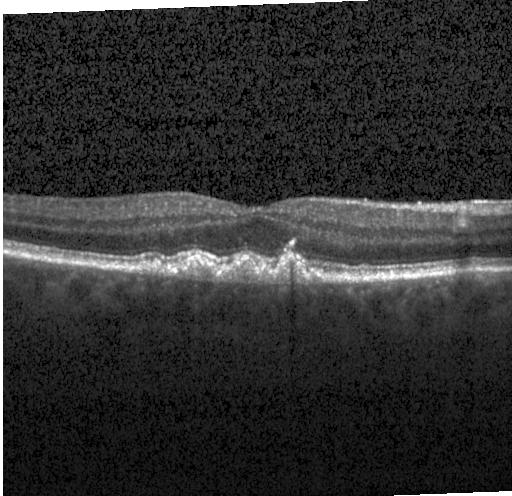
Optical coherence tomography B-scan · macular scan · spectral-domain OCT — Diagnosis: drusen.